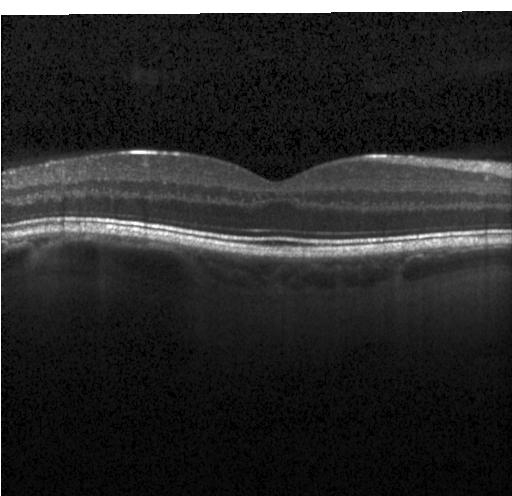

This B-scan demonstrates no evidence of CNV, DME, or drusen.